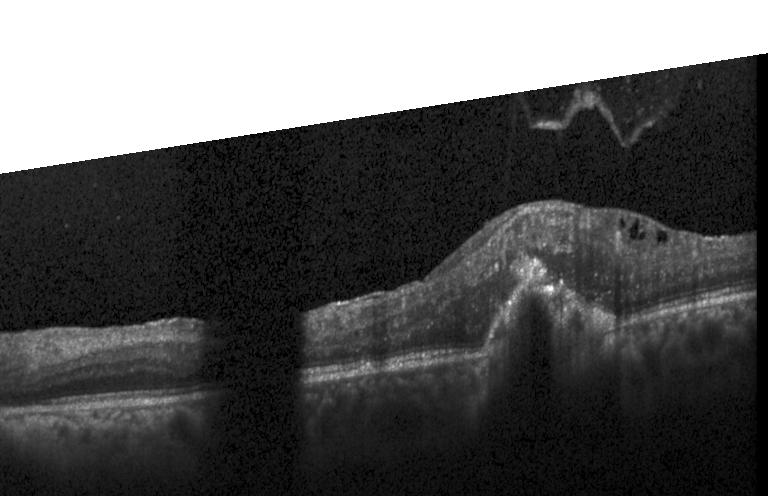 Acquired on a Heidelberg Spectralis · OCT B-scan · spectral-domain OCT.
Diagnosis: choroidal neovascularization.